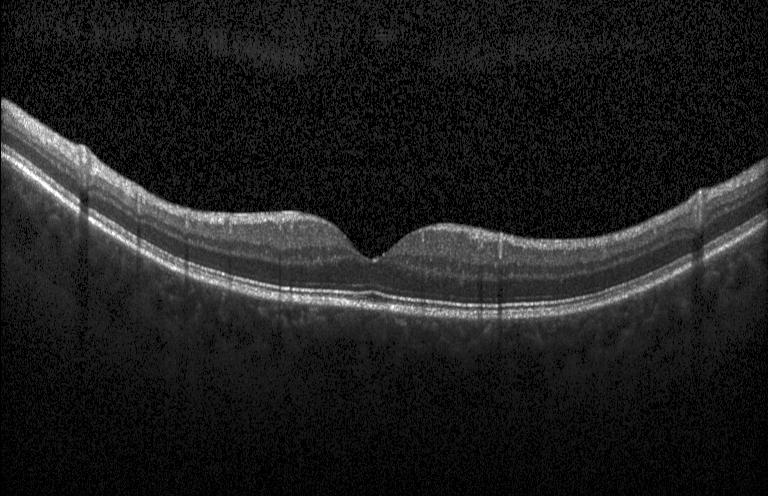
Retinal OCT B-scan
The scan shows neither choroidal neovascularization, diabetic macular edema, nor drusen.